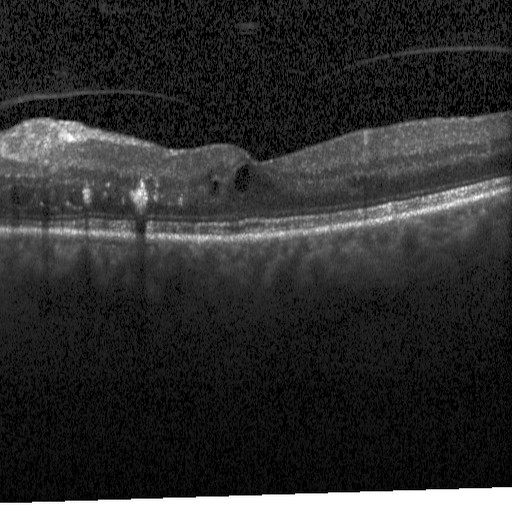

Spectral-domain OCT B-scan: diabetic macular edema (DME).